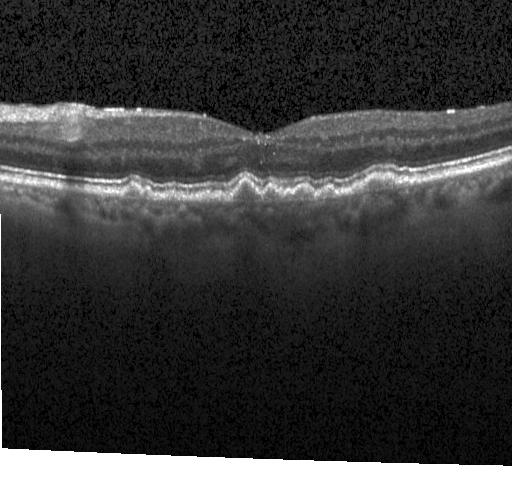 Optical coherence tomography scan
Dx: sub-RPE drusenoid deposits.